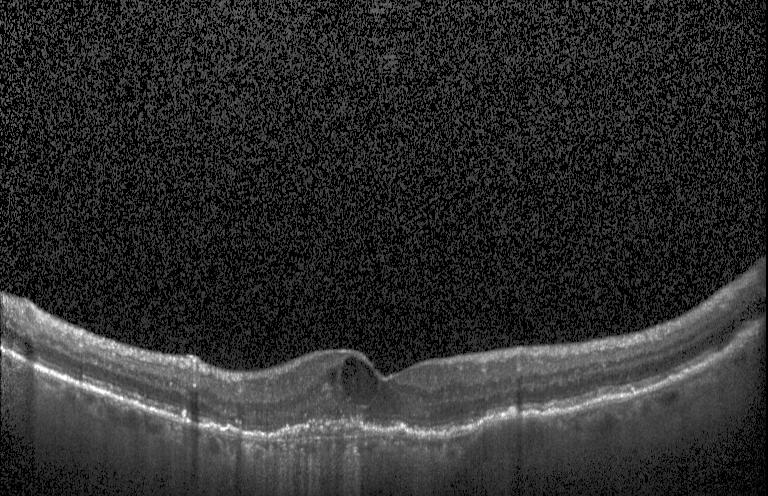
Macular OCT: CNV.